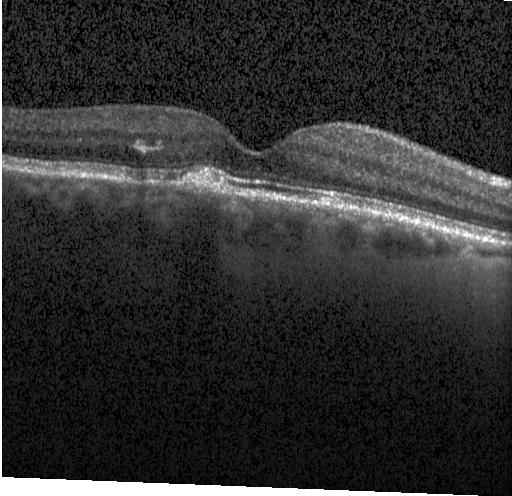
Through the macula. OCT line scan. Acquired on a Heidelberg Spectralis. Spectral-domain optical coherence tomography. Diagnosis: sub-RPE drusenoid deposits.